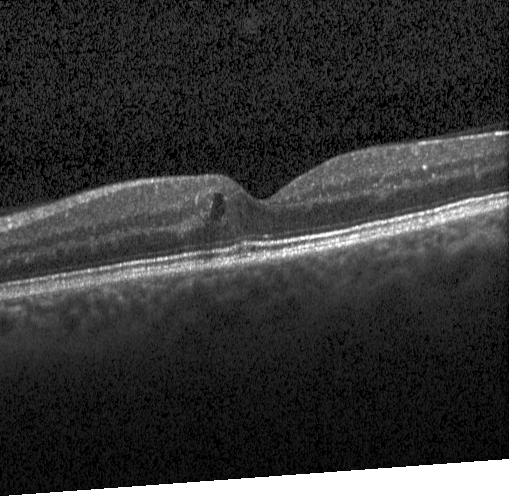
Instrument: Heidelberg Spectralis · retinal OCT cross-section · horizontal scan through the fovea — Diabetic macular edema (DME).